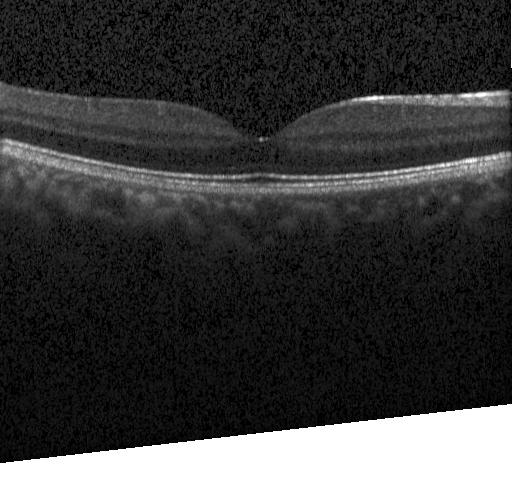

Optical coherence tomography scan · acquired on a Heidelberg Spectralis · spectral-domain optical coherence tomography · centered on the fovea
Macular OCT: neither CNV, DME, nor drusen.